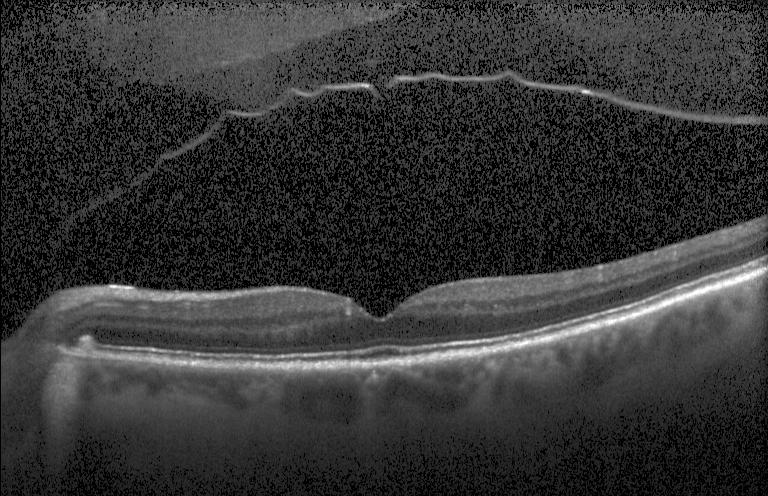
Retinal OCT cross-section.
No evidence of choroidal neovascularization, diabetic macular edema, or drusen.